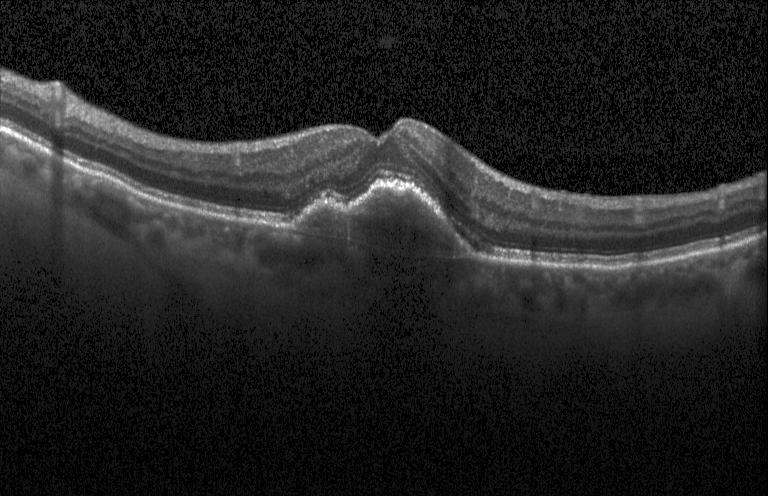
Acquired on a Heidelberg Spectralis; spectral-domain optical coherence tomography; optical coherence tomography scan; through the macula — This B-scan demonstrates choroidal neovascularization.